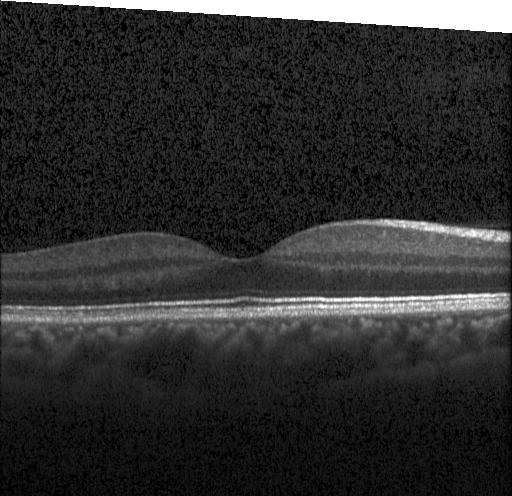

No CNV, no DME, and no drusen.